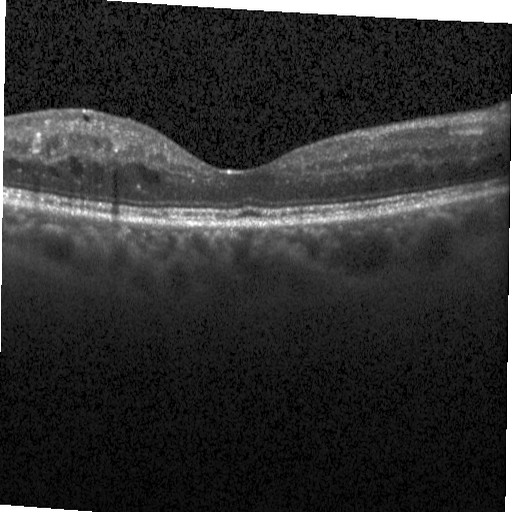
SD-OCT. Instrument: Heidelberg Spectralis. Optical coherence tomography B-scan. Dx: diabetic macular edema (DME).